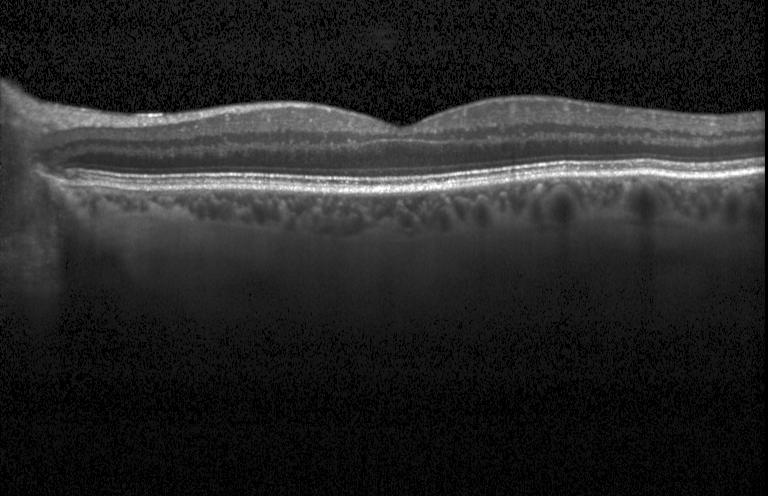 Macular scan. OCT line scan.
Dx: no choroidal neovascularization, no diabetic macular edema, and no drusen.